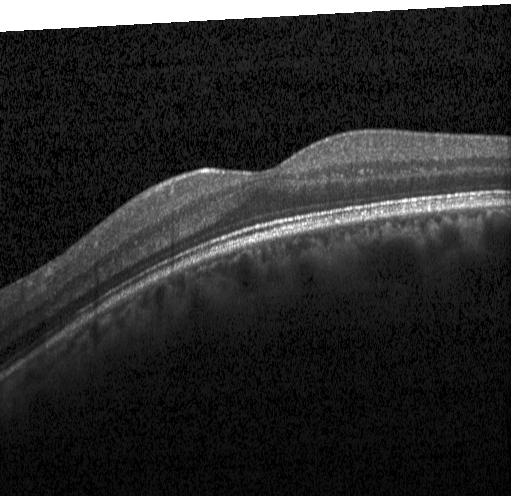 Finding: no choroidal neovascularization, diabetic macular edema, or drusen.